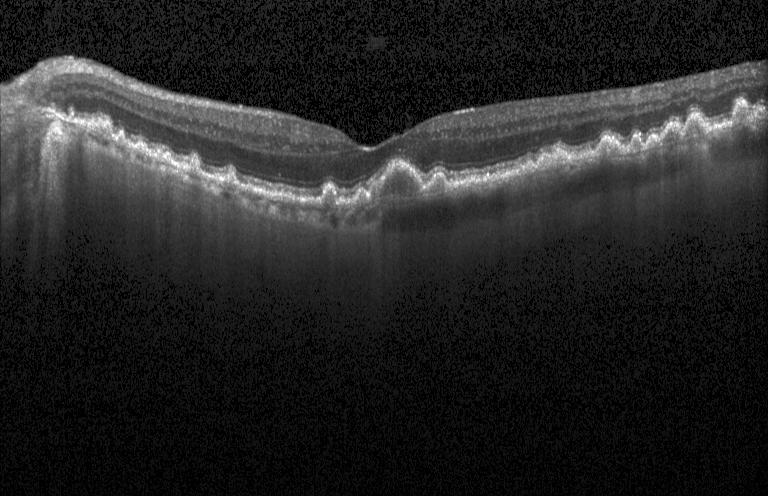 Retinal OCT cross-section showing sub-RPE drusenoid deposits.